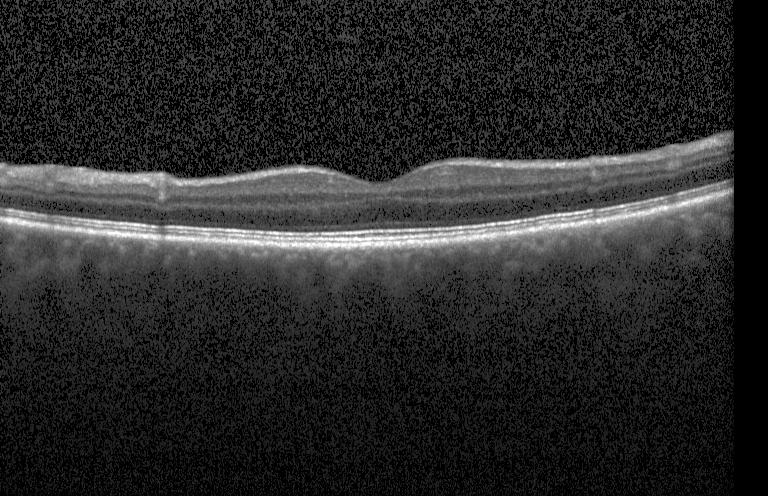

OCT scan showing neither choroidal neovascularization, diabetic macular edema, nor drusen.